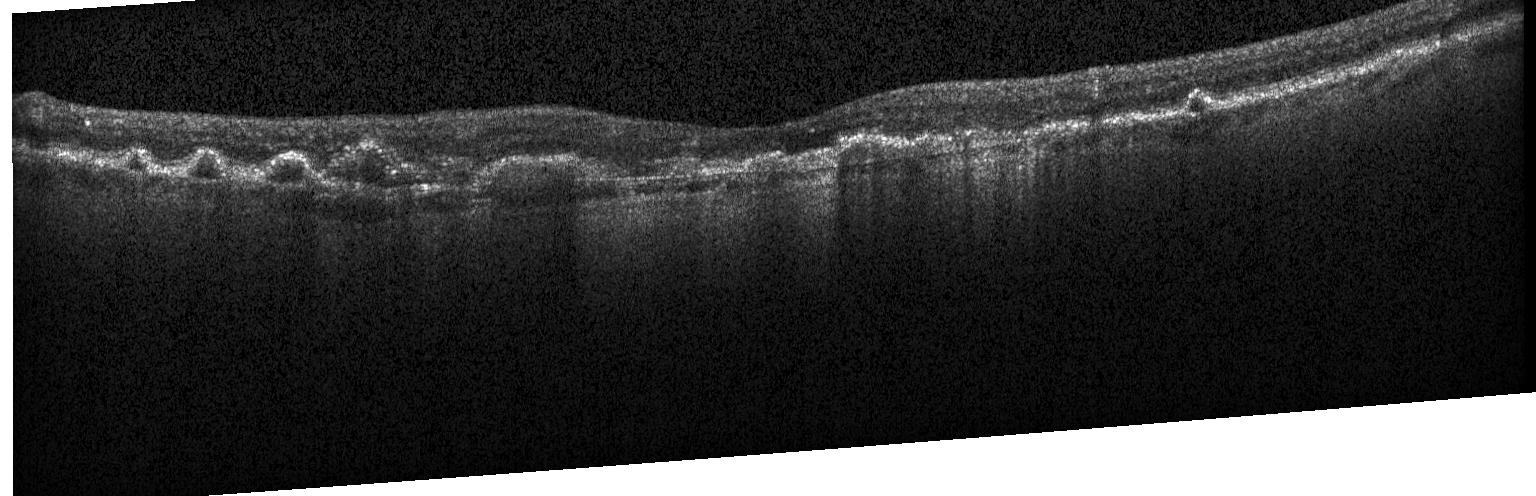

Retinal OCT B-scan · spectral-domain optical coherence tomography
Macular OCT: CNV.